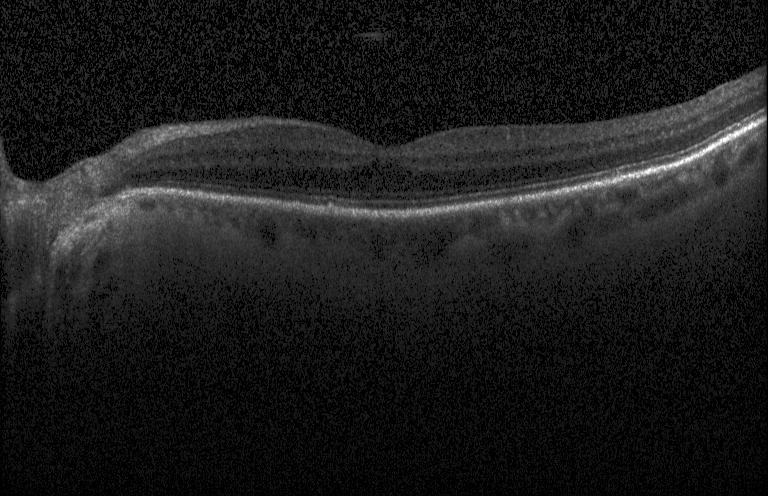 Macular scan · optical coherence tomography B-scan · SD-OCT. Diagnosis: neither CNV, DME, nor drusen.